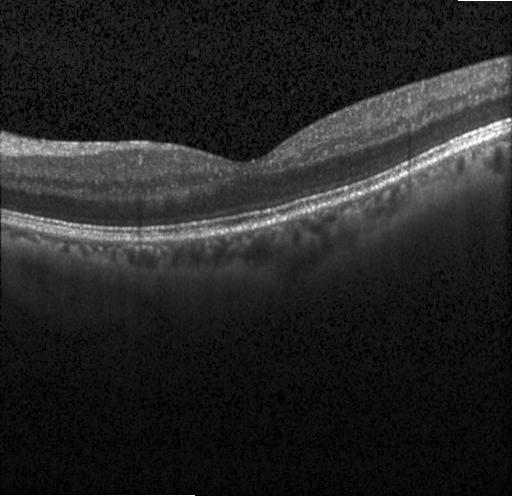
Fovea-centered, OCT line scan.
This B-scan demonstrates no choroidal neovascularization, diabetic macular edema, or drusen.